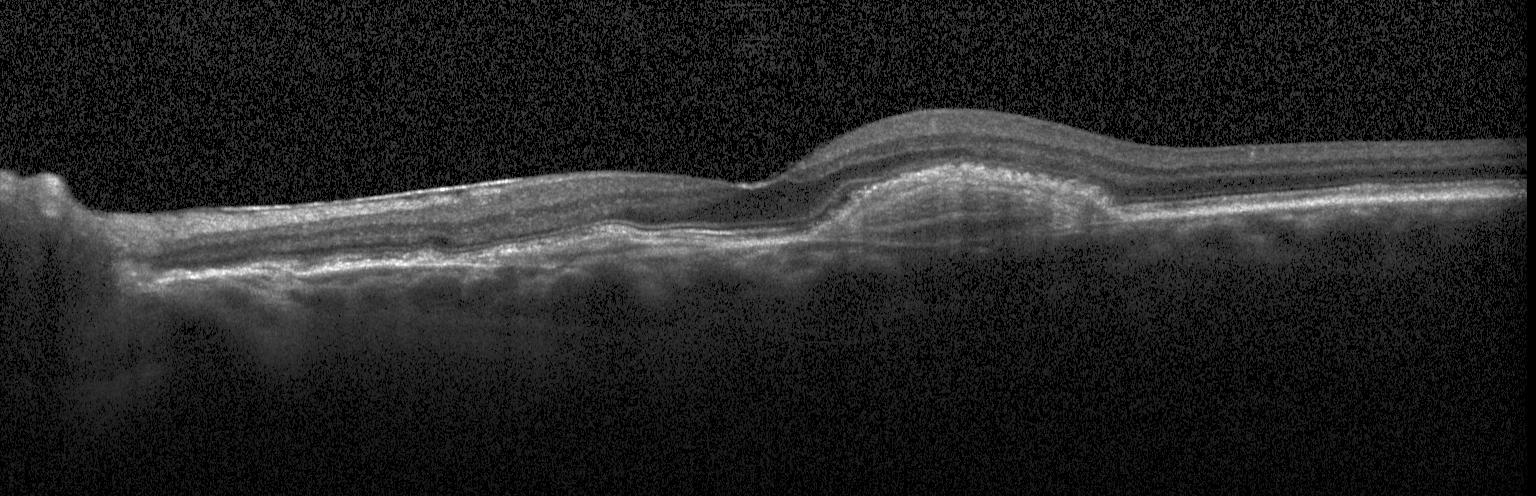

Fovea-centered. Retinal OCT B-scan. Instrument: Heidelberg Spectralis
Diagnosis: choroidal neovascularization.